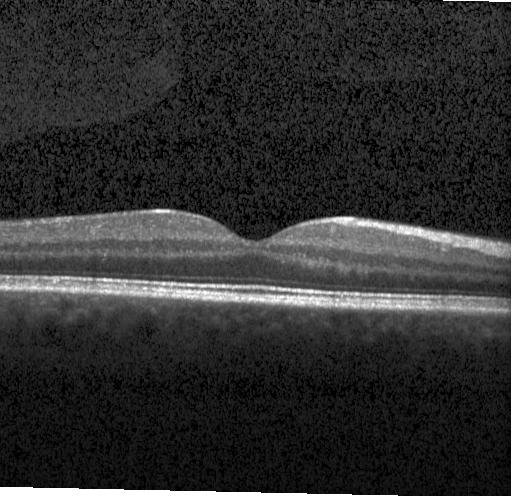 SD-OCT, OCT B-scan
Diagnosis: no evidence of choroidal neovascularization, diabetic macular edema, or drusen.